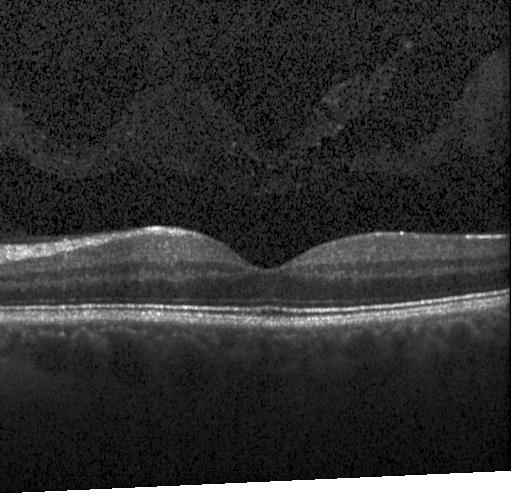 OCT scan showing no choroidal neovascularization, no diabetic macular edema, and no drusen.